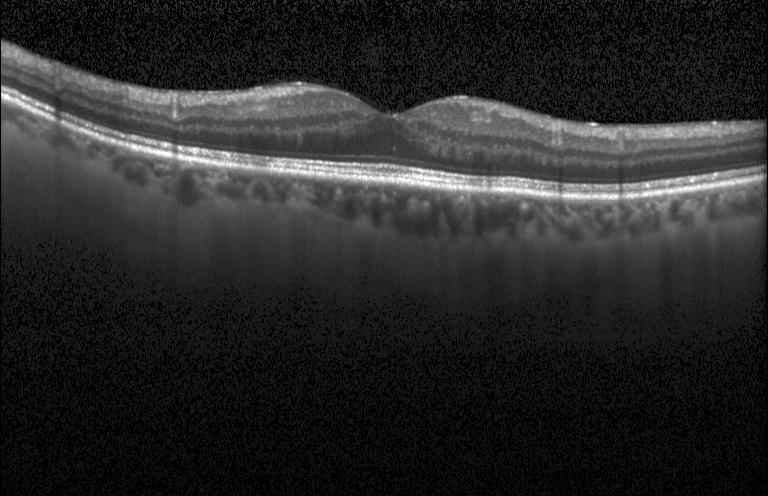
Diagnosis: neither choroidal neovascularization, diabetic macular edema, nor drusen.